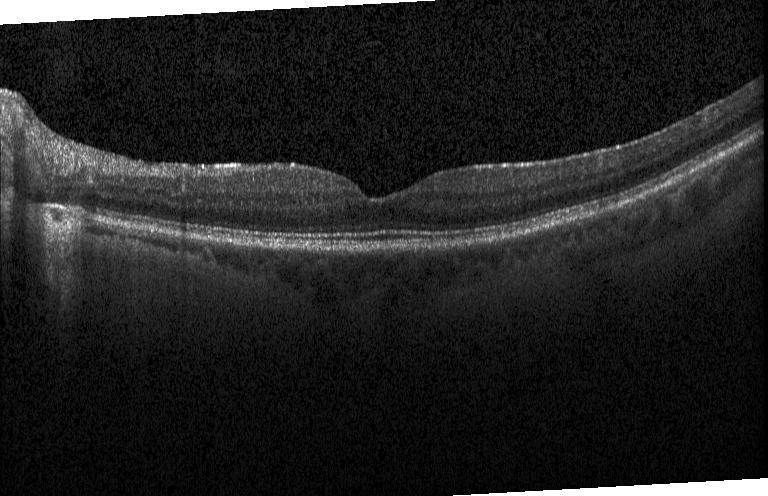
Retinal OCT cross-section showing no evidence of choroidal neovascularization, diabetic macular edema, or drusen.